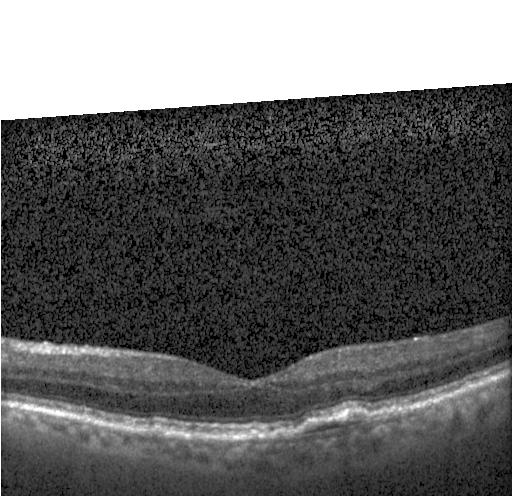
Fovea-centered · OCT B-scan. Impression: a choroidal neovascular membrane.